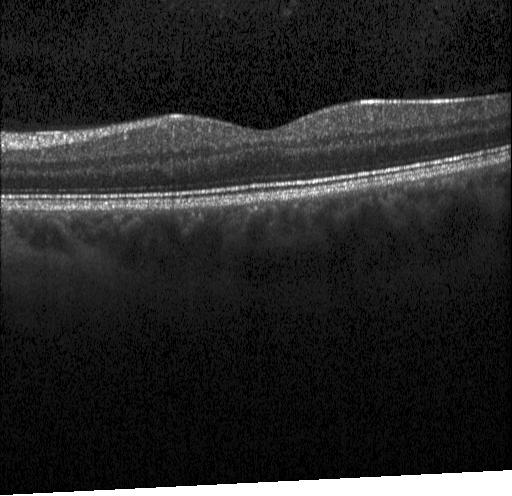
OCT scan showing neither choroidal neovascularization, diabetic macular edema, nor drusen.